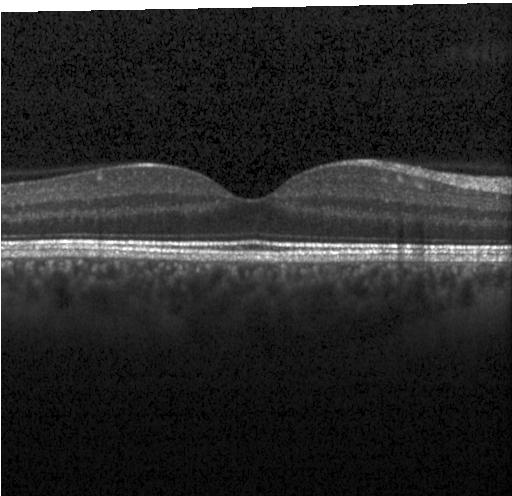 Diagnosis: no choroidal neovascularization, diabetic macular edema, or drusen.